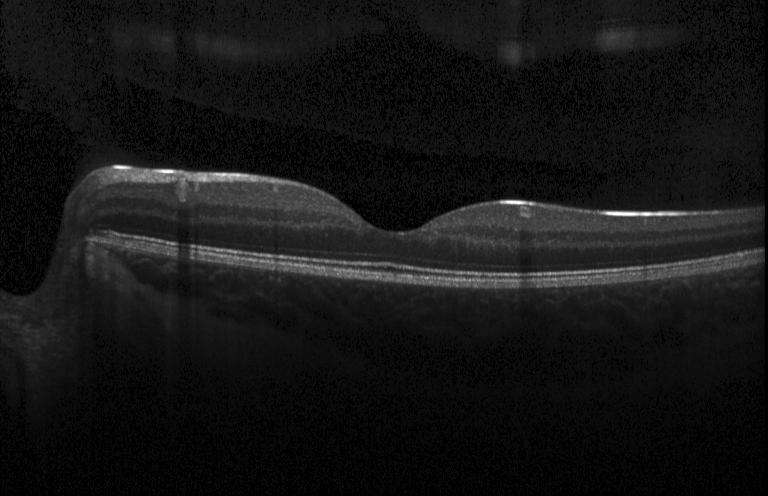
Dx: neither choroidal neovascularization, diabetic macular edema, nor drusen.